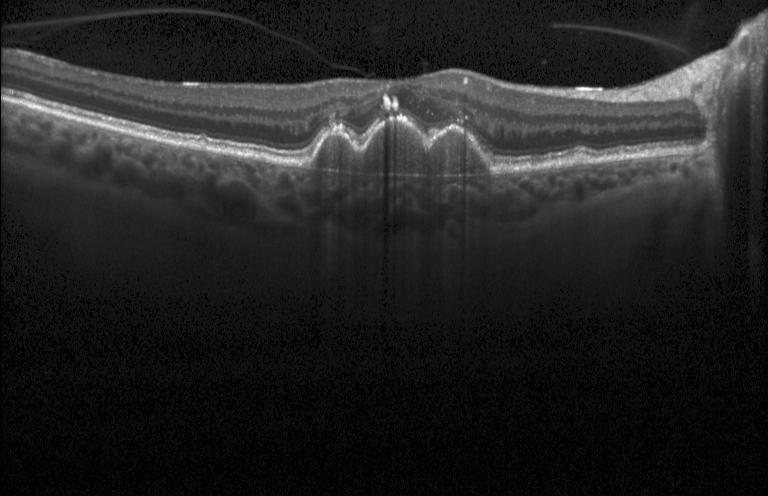
Macular OCT demonstrating a choroidal neovascular membrane.